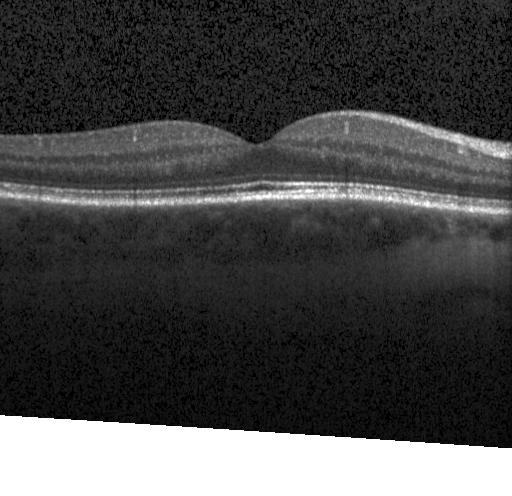 Horizontal scan through the fovea, optical coherence tomography scan, Heidelberg Spectralis. Impression: no evidence of choroidal neovascularization, diabetic macular edema, or drusen.